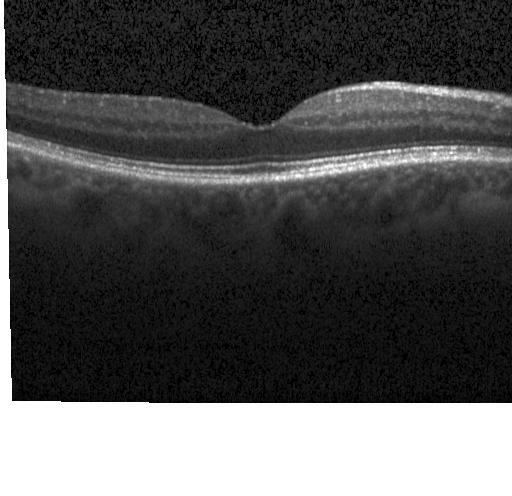
Retinal OCT cross-section.
No evidence of choroidal neovascularization, diabetic macular edema, or drusen.